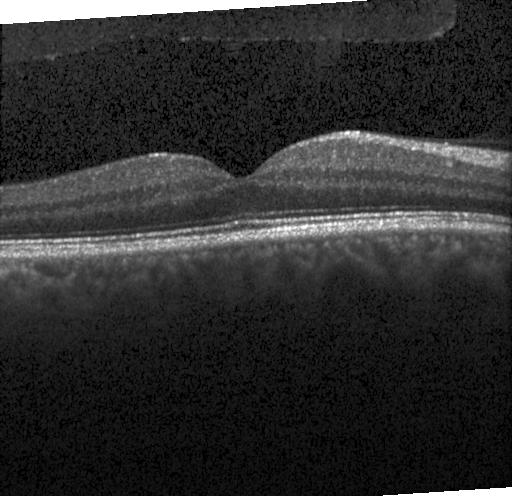

Diagnosis: neither choroidal neovascularization, diabetic macular edema, nor drusen.